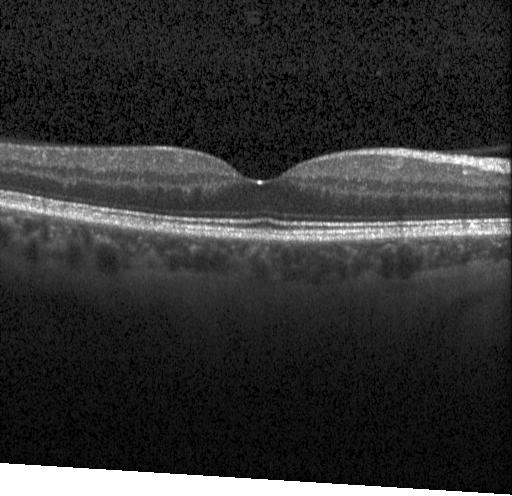

Spectral-domain OCT, retinal OCT B-scan.
The scan shows no evidence of CNV, DME, or drusen.